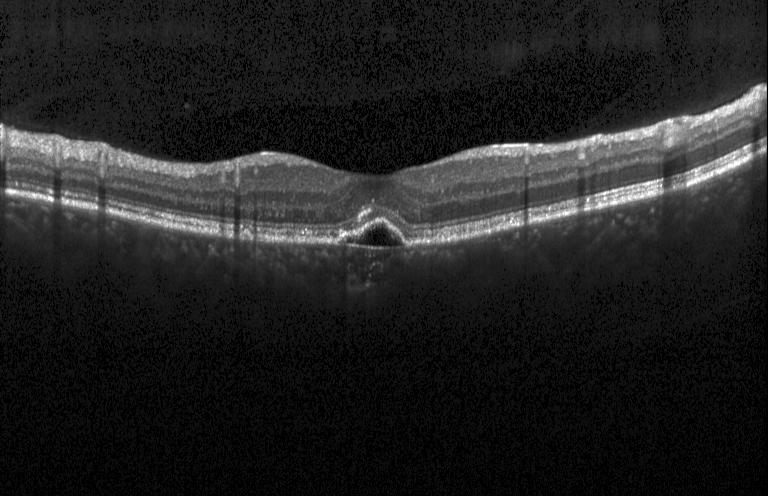 Optical coherence tomography scan — Impression: choroidal neovascularization (CNV).